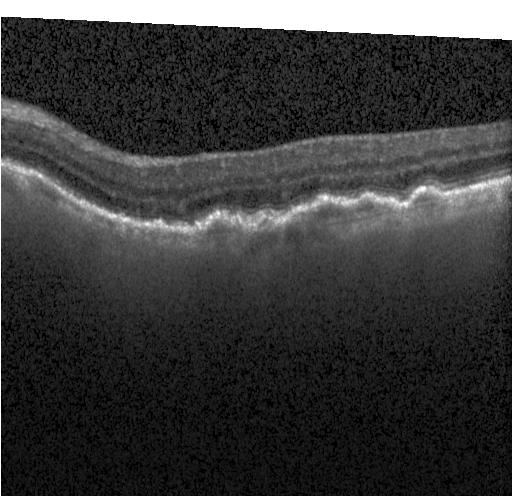
OCT B-scan, SD-OCT, fovea-centered — Macular OCT: choroidal neovascularization (CNV).